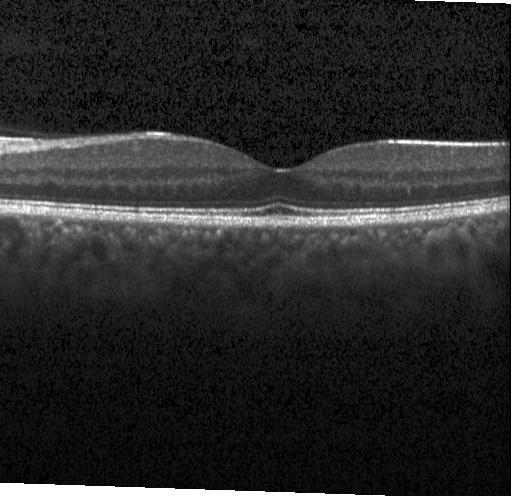 Macular OCT demonstrating no choroidal neovascularization, no diabetic macular edema, and no drusen.